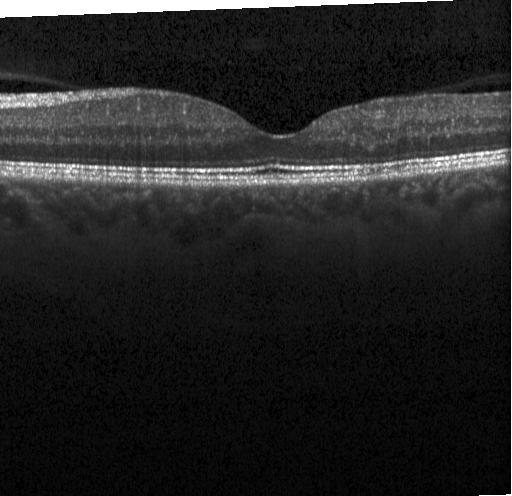 Dx: no choroidal neovascularization, no diabetic macular edema, and no drusen.